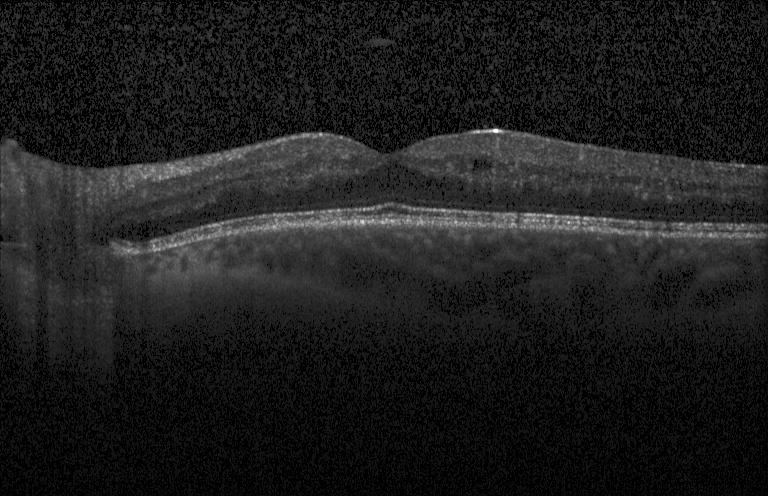 OCT line scan · SD-OCT · instrument: Heidelberg Spectralis · fovea-centered. The scan shows diabetic macular edema.